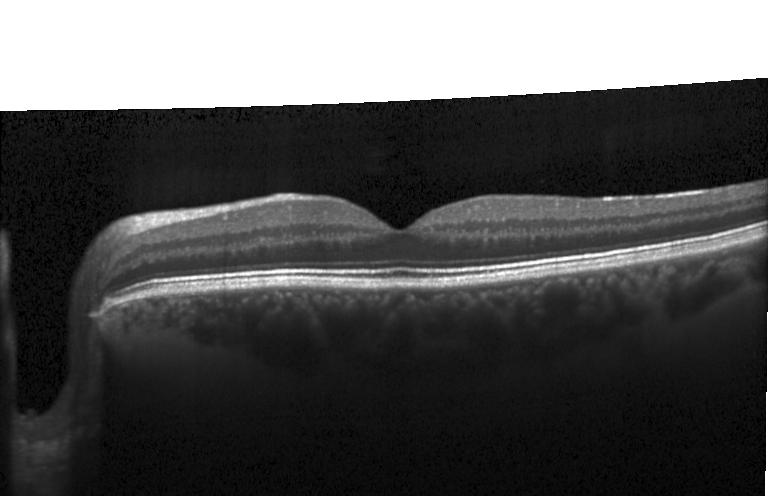
Horizontal scan through the fovea · Heidelberg Spectralis · optical coherence tomography scan.
Finding: no evidence of choroidal neovascularization, diabetic macular edema, or drusen.